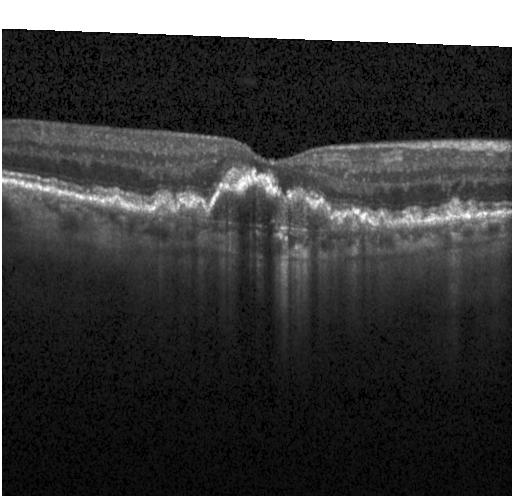 Macular OCT: CNV.